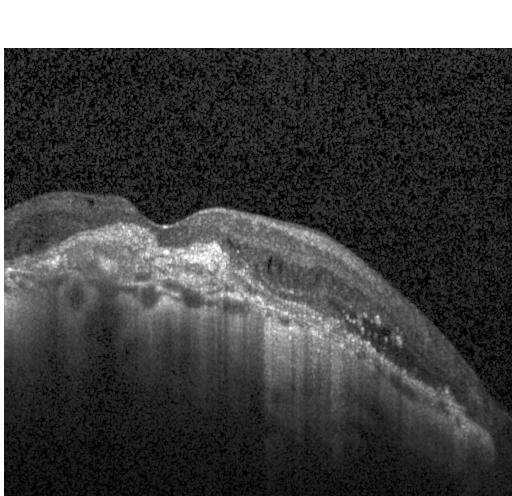
Spectral-domain optical coherence tomography; optical coherence tomography scan
A choroidal neovascular membrane.